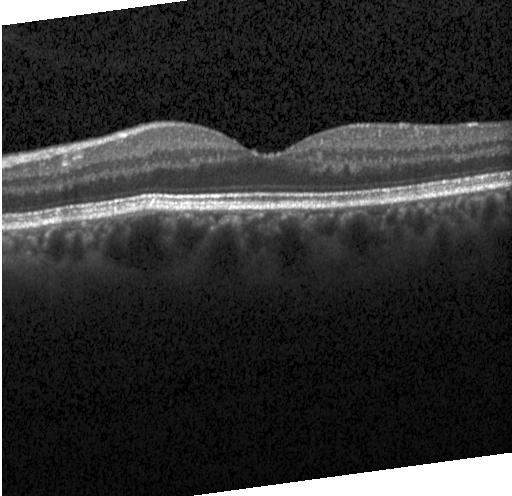 OCT scan showing neither choroidal neovascularization, diabetic macular edema, nor drusen.